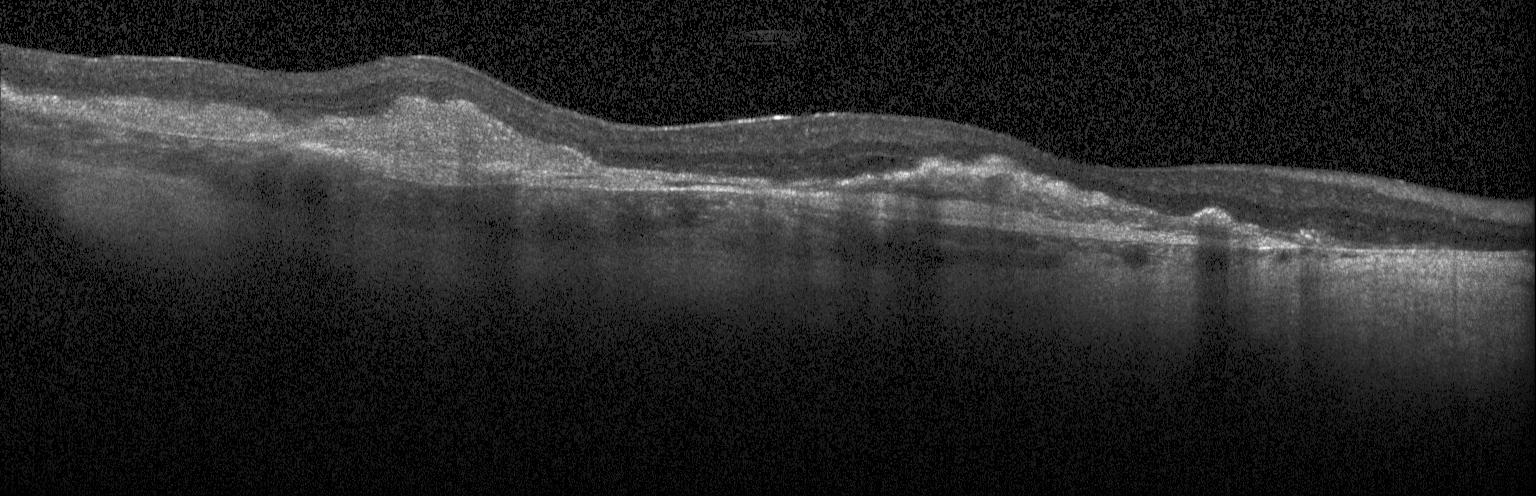
OCT scan showing CNV.